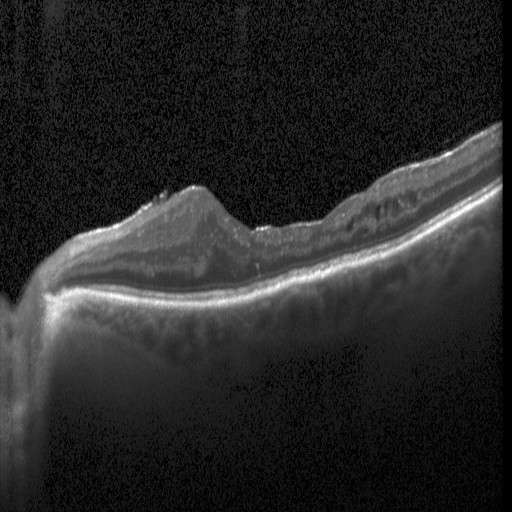 OCT B-scan showing DME.